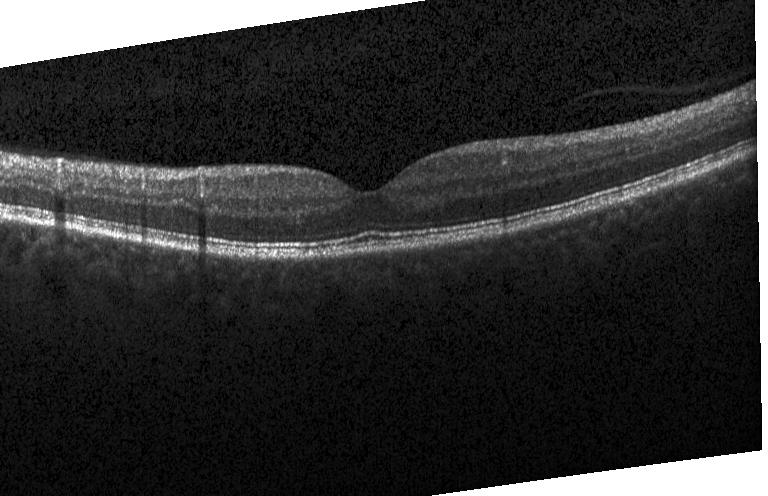

Retinal OCT cross-section; acquired on a Heidelberg Spectralis; spectral-domain optical coherence tomography. Assessment: no evidence of choroidal neovascularization, diabetic macular edema, or drusen.